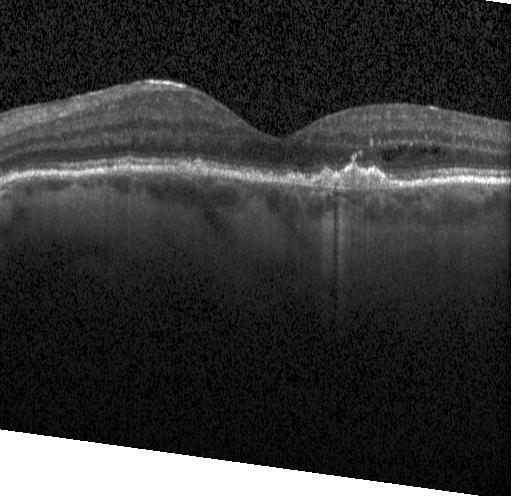

OCT B-scan.
The scan shows sub-RPE drusenoid deposits.